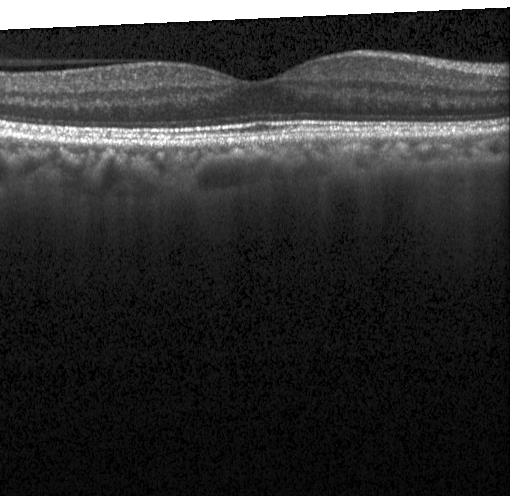 Optical coherence tomography scan · horizontal scan through the fovea
Macular OCT: no choroidal neovascularization, diabetic macular edema, or drusen.